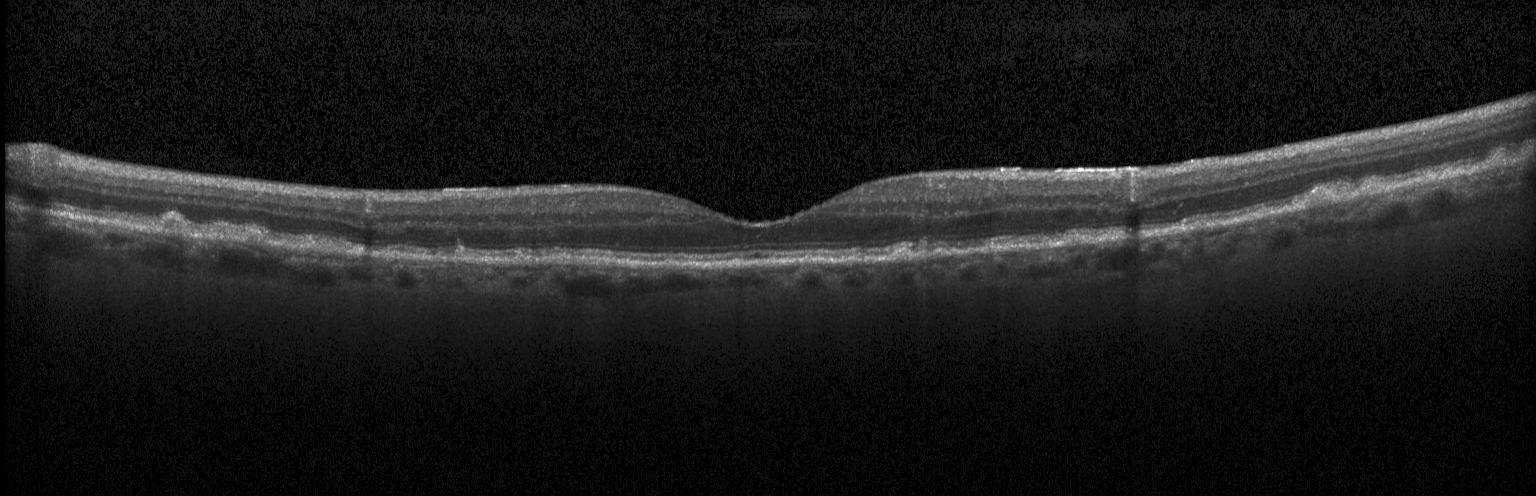 Optical coherence tomography scan. Drusen.